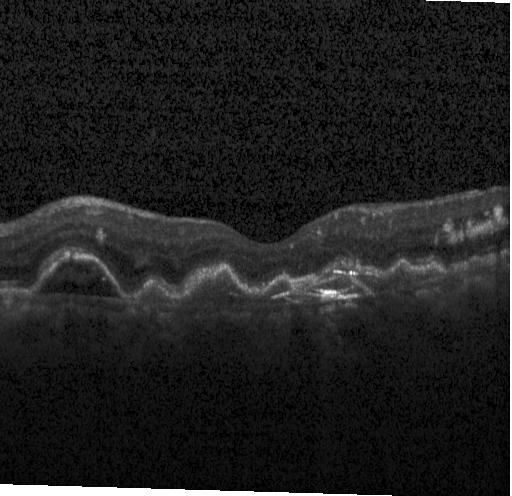
Macular OCT demonstrating choroidal neovascularization (CNV).